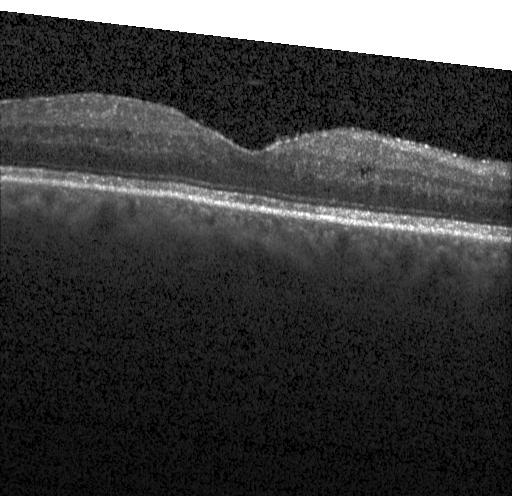

Impression: no evidence of CNV, DME, or drusen.